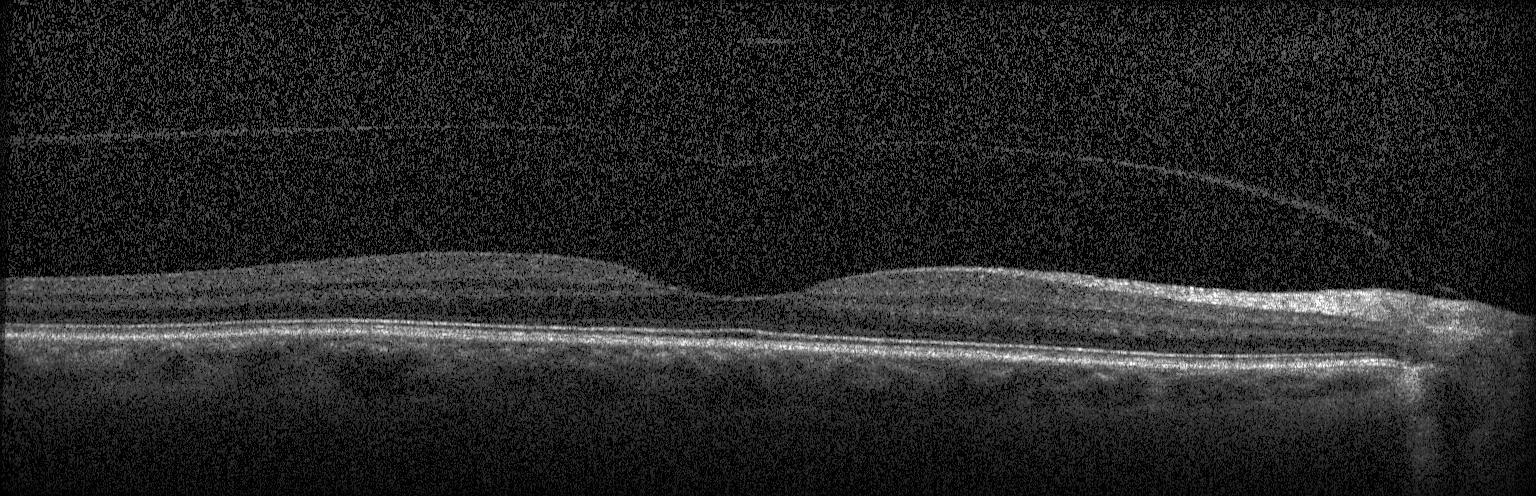
Acquired on a Heidelberg Spectralis. Spectral-domain optical coherence tomography. Macular scan. OCT B-scan. Macular OCT: no choroidal neovascularization, no diabetic macular edema, and no drusen.